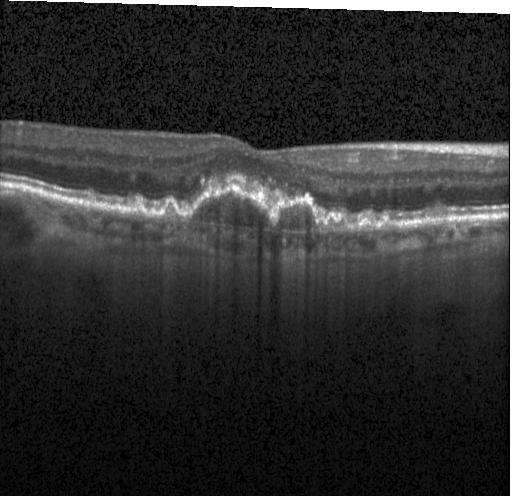 Heidelberg Spectralis OCT system, SD-OCT, OCT B-scan — Choroidal neovascularization (CNV).